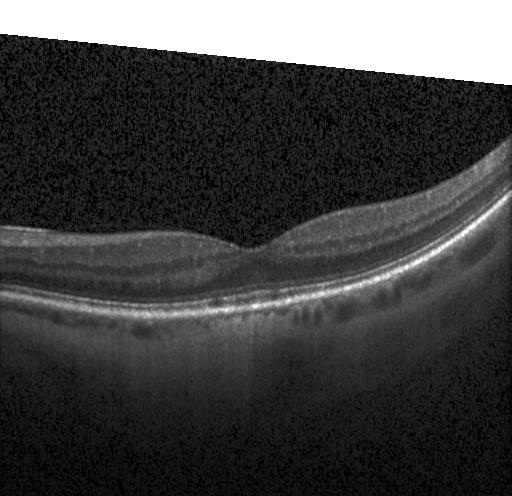 Spectral-domain optical coherence tomography; OCT B-scan — Finding: no CNV, no DME, and no drusen.